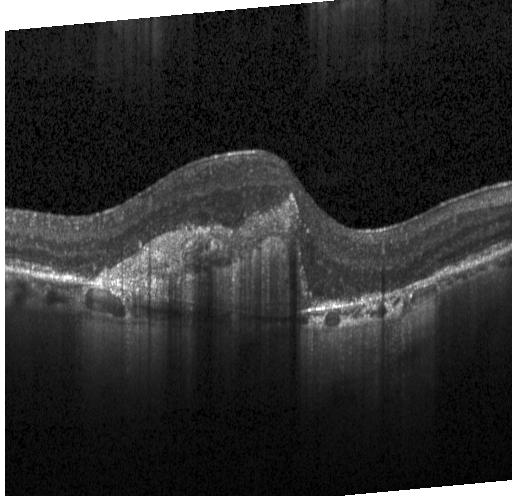

Through the macula. SD-OCT. Retinal OCT B-scan. Acquired on a Heidelberg Spectralis — Diagnosis: CNV.